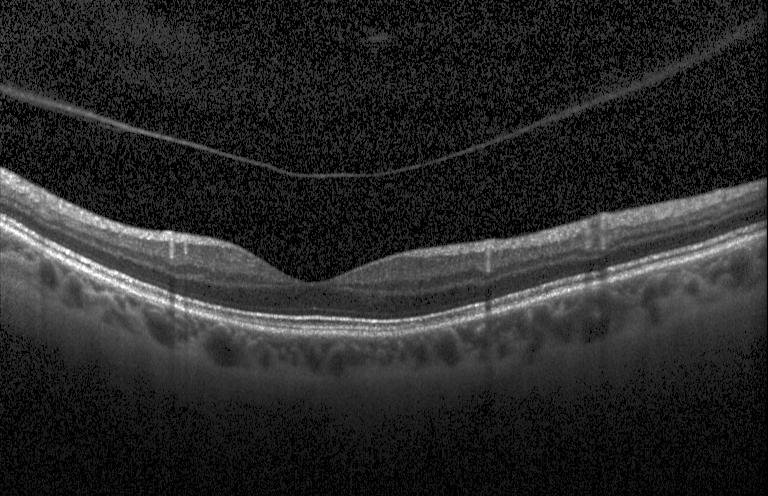 OCT B-scan · instrument: Heidelberg Spectralis · SD-OCT · through the macula
Diagnosis: no choroidal neovascularization, no diabetic macular edema, and no drusen.